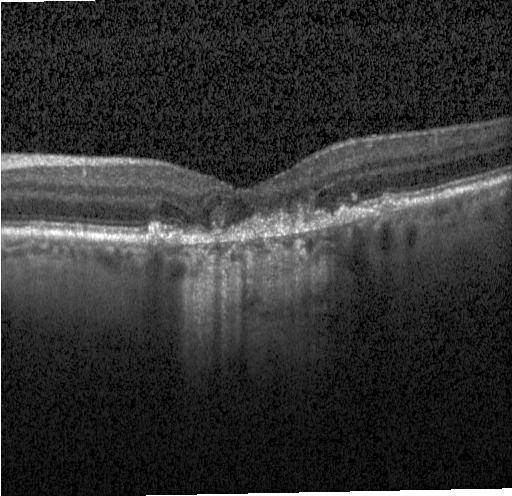 OCT B-scan · spectral-domain OCT — Finding: a choroidal neovascular membrane.